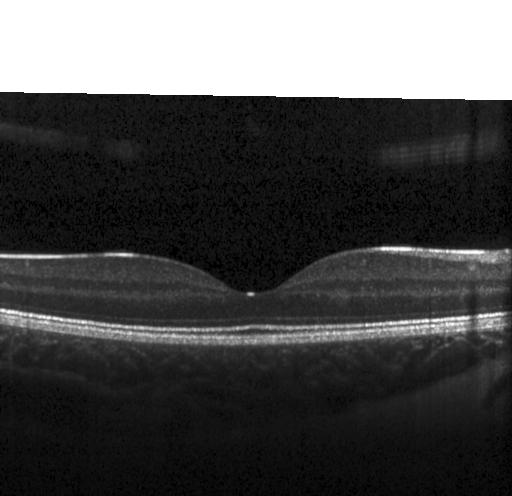

No choroidal neovascularization, diabetic macular edema, or drusen.